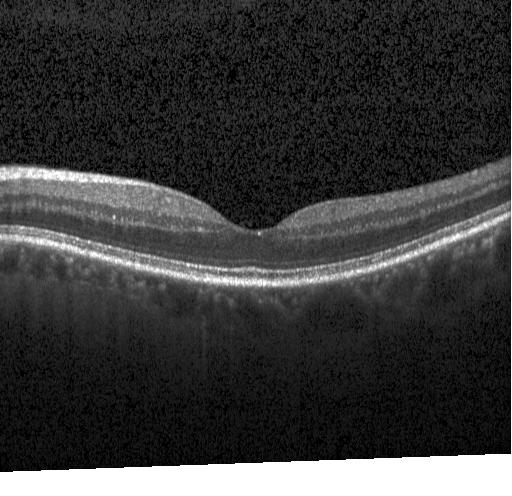

OCT B-scan · centered on the fovea. Assessment: no choroidal neovascularization, no diabetic macular edema, and no drusen.